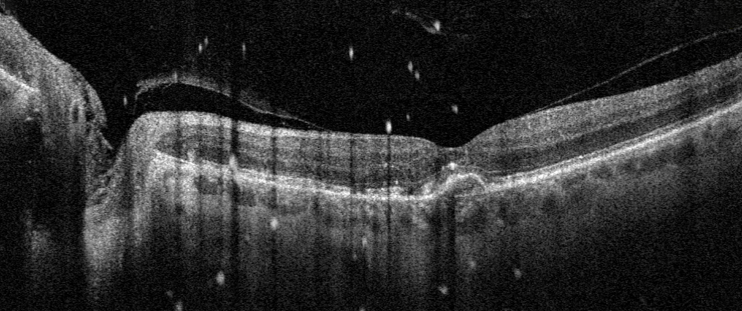 Retinal OCT cross-section. Diagnosis: age-related macular degeneration (AMD).